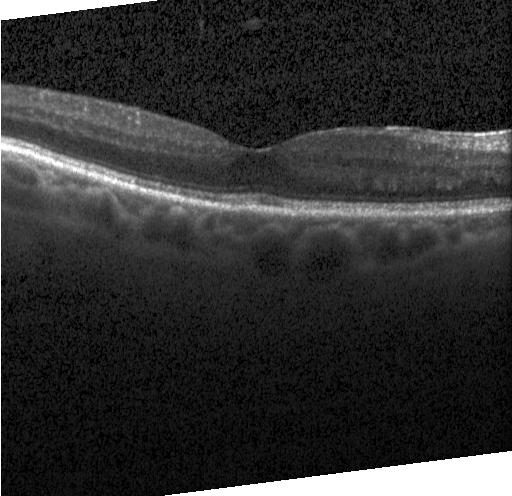

Optical coherence tomography scan — Finding: no evidence of CNV, DME, or drusen.